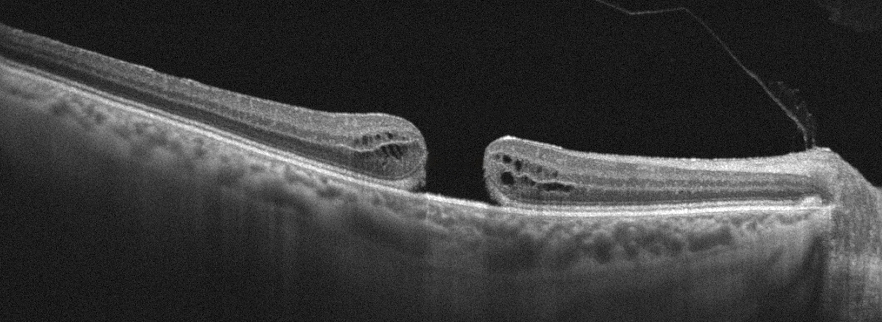 Macular scan · Optovue Avanti RTVue XR · retinal OCT cross-section · oculus dexter — Assessment: vitreomacular interface disease (VID).